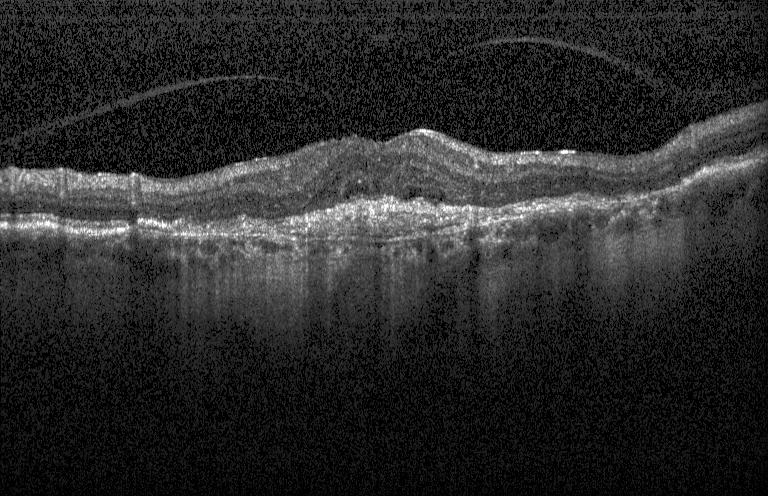 Acquired on a Heidelberg Spectralis; spectral-domain optical coherence tomography; optical coherence tomography scan.
Impression: a choroidal neovascular membrane.